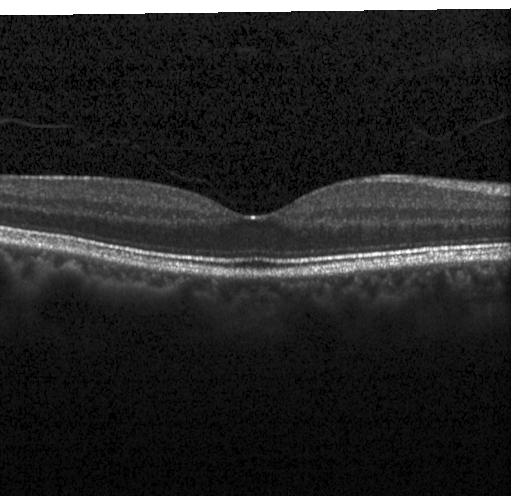
SD-OCT · optical coherence tomography scan · horizontal scan through the fovea.
Diagnosis: no choroidal neovascularization, diabetic macular edema, or drusen.